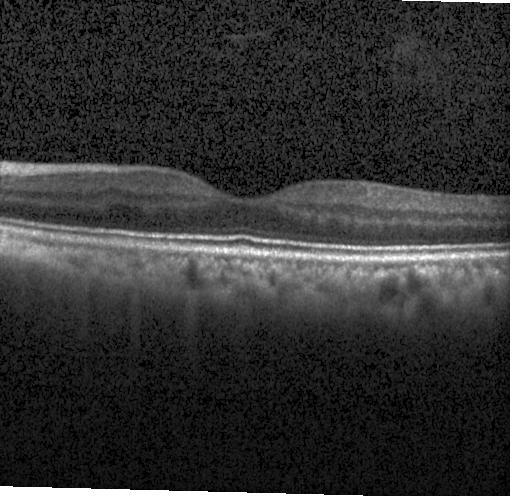 Spectral-domain OCT, Heidelberg Spectralis, optical coherence tomography B-scan
The scan shows no evidence of CNV, DME, or drusen.